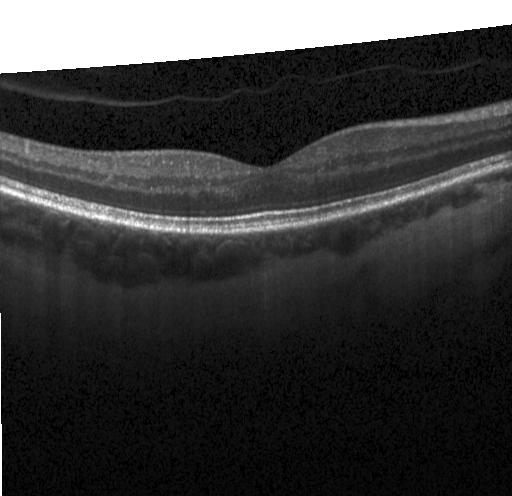

The scan shows neither choroidal neovascularization, diabetic macular edema, nor drusen.